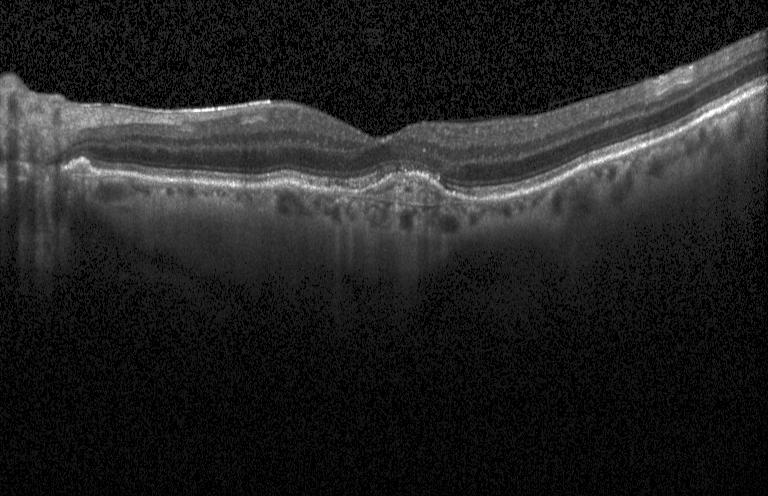
OCT B-scan · fovea-centered. Finding: a choroidal neovascular membrane.